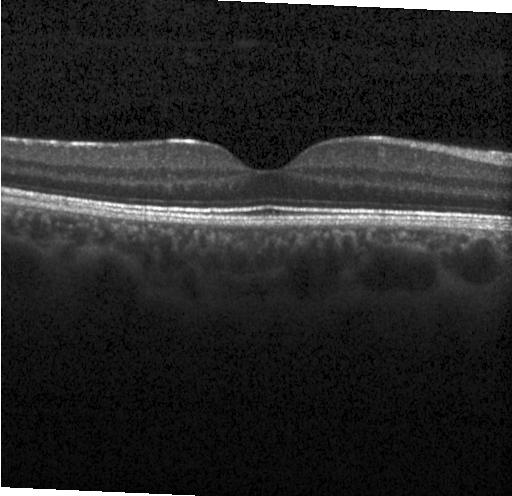

Spectral-domain OCT · retinal OCT B-scan.
Diagnosis: no evidence of choroidal neovascularization, diabetic macular edema, or drusen.